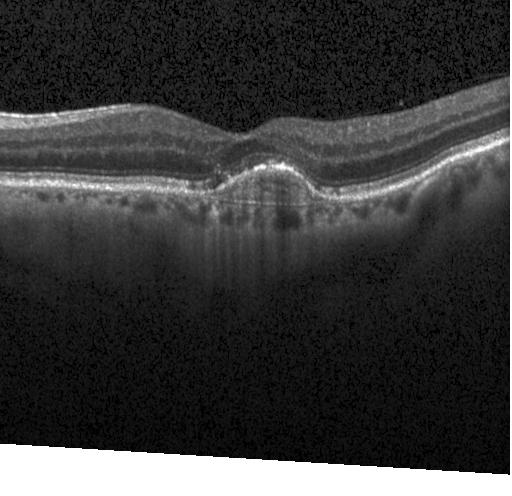
Spectral-domain optical coherence tomography, retinal OCT cross-section. Assessment: a choroidal neovascular membrane.